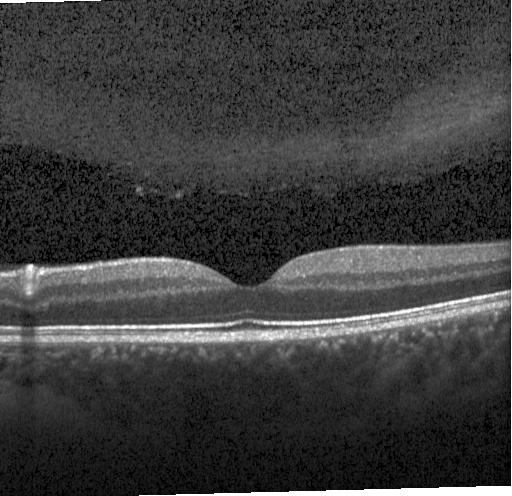 OCT line scan, macular scan. Assessment: neither choroidal neovascularization, diabetic macular edema, nor drusen.